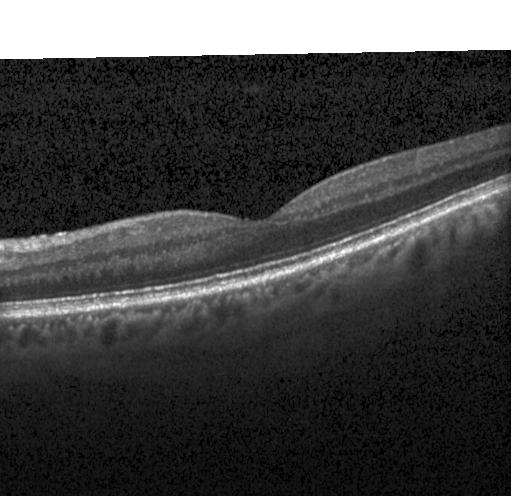 Spectral-domain OCT; OCT B-scan — Finding: no evidence of choroidal neovascularization, diabetic macular edema, or drusen.